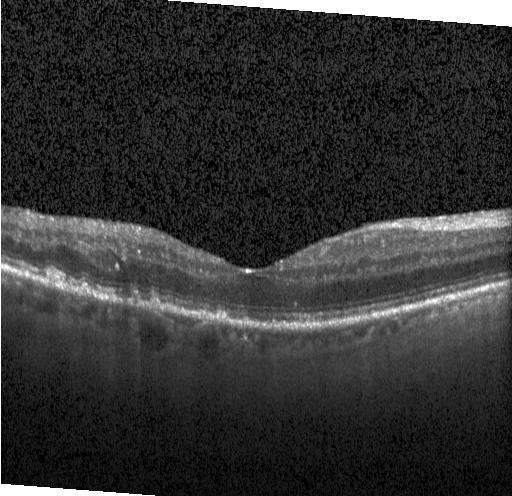 SD-OCT; through the macula; optical coherence tomography scan.
Assessment: sub-RPE drusenoid deposits.